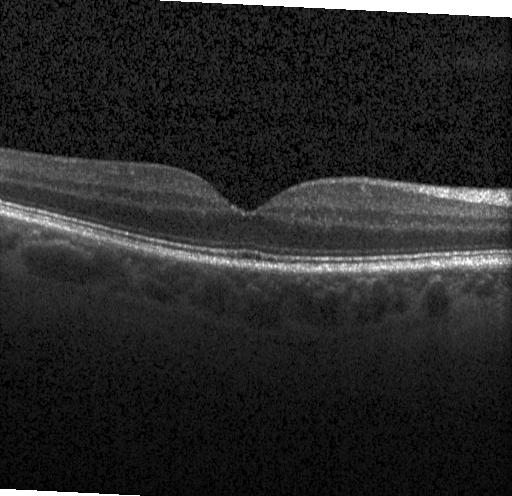
Neither choroidal neovascularization, diabetic macular edema, nor drusen.